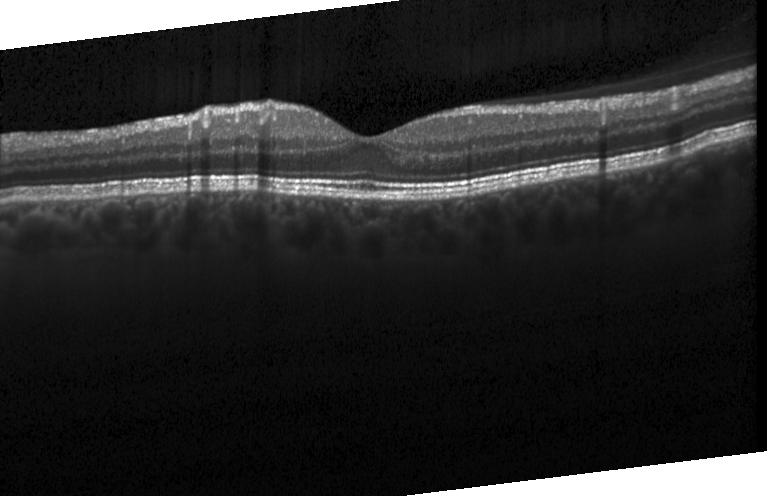 Macular OCT: neither choroidal neovascularization, diabetic macular edema, nor drusen.